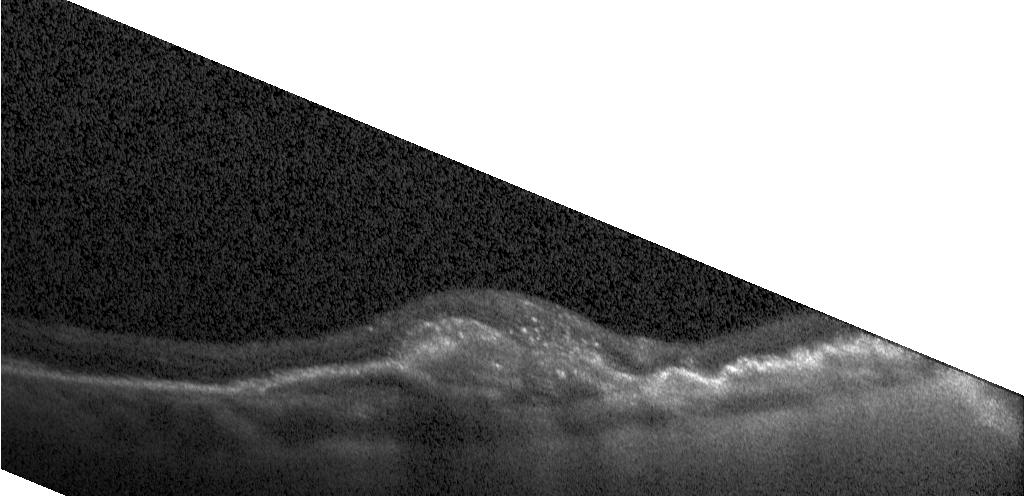
Optical coherence tomography B-scan — Impression: choroidal neovascularization.